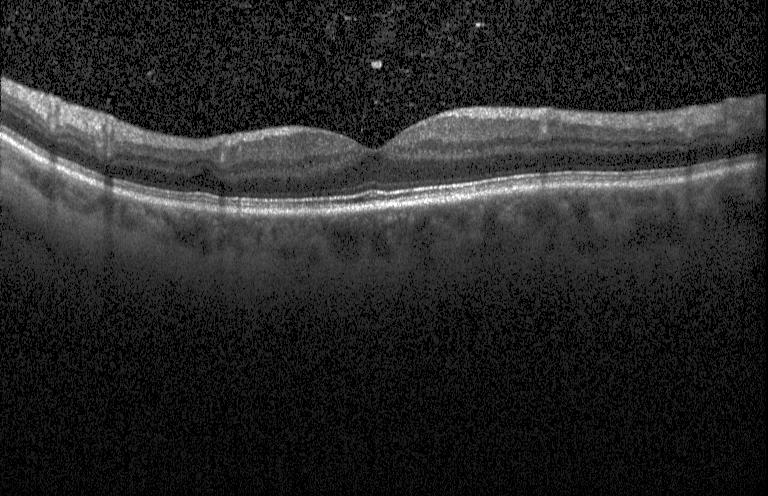 Dx: no evidence of CNV, DME, or drusen.